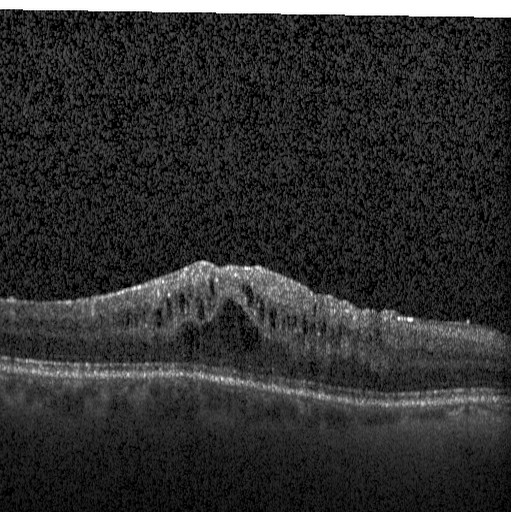

Assessment: DME.